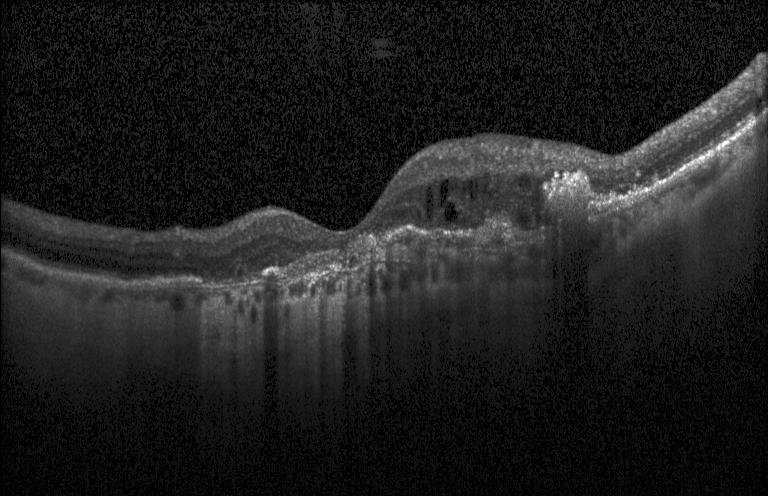 Retinal OCT B-scan · Heidelberg Spectralis.
Diagnosis: choroidal neovascularization.